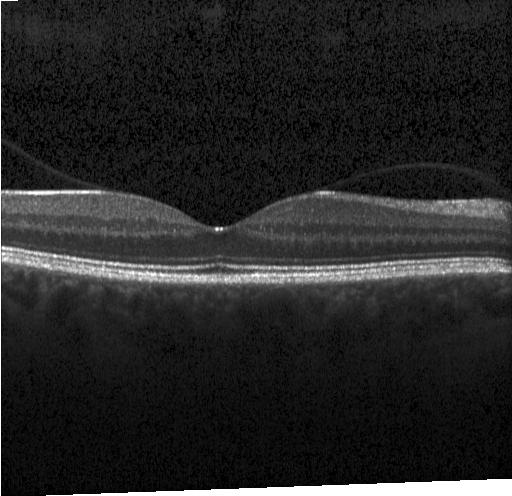

OCT finding: no choroidal neovascularization, no diabetic macular edema, and no drusen.